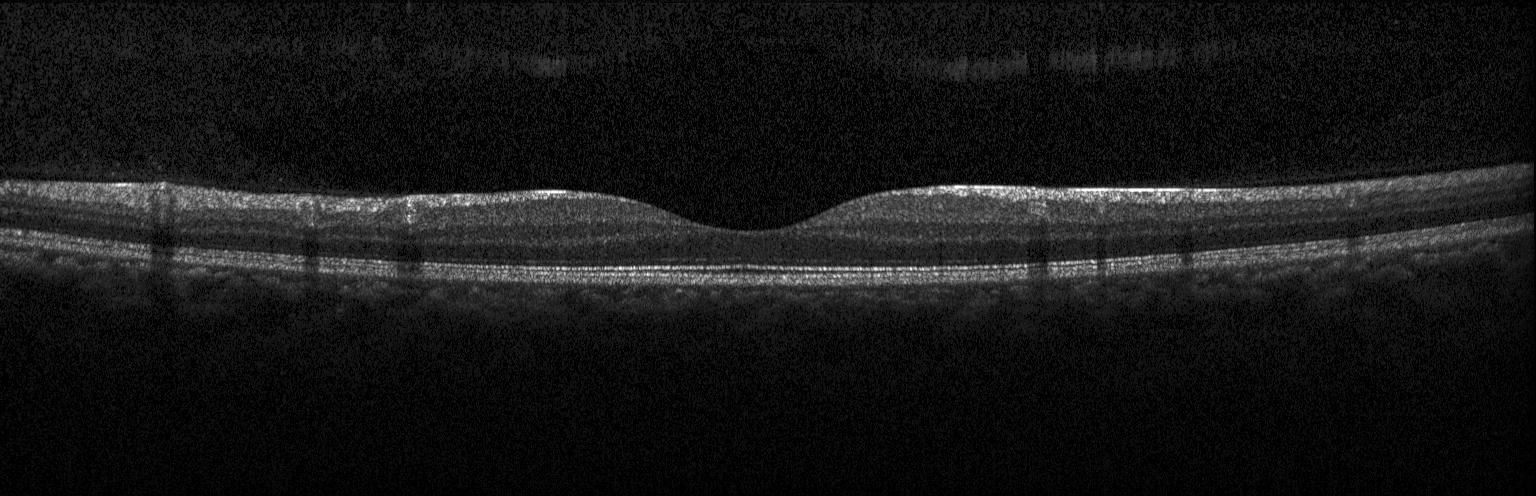

Finding: no choroidal neovascularization, diabetic macular edema, or drusen.